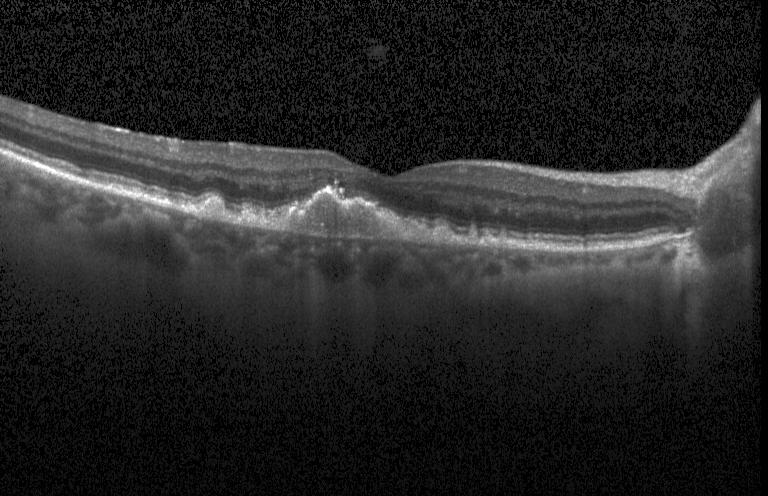
OCT line scan; through the macula; SD-OCT
Impression: choroidal neovascularization.